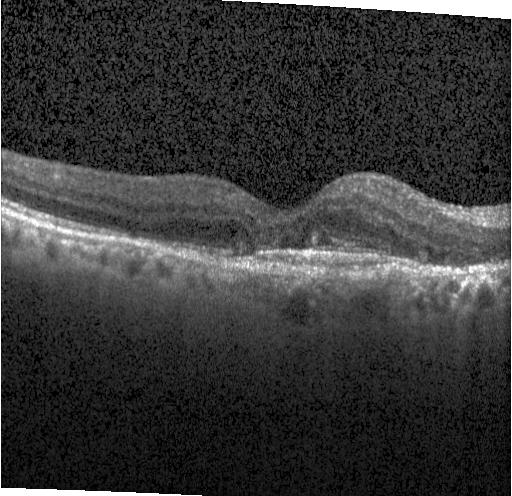

Heidelberg Spectralis, through the macula, OCT B-scan, SD-OCT. Diagnosis: choroidal neovascularization.